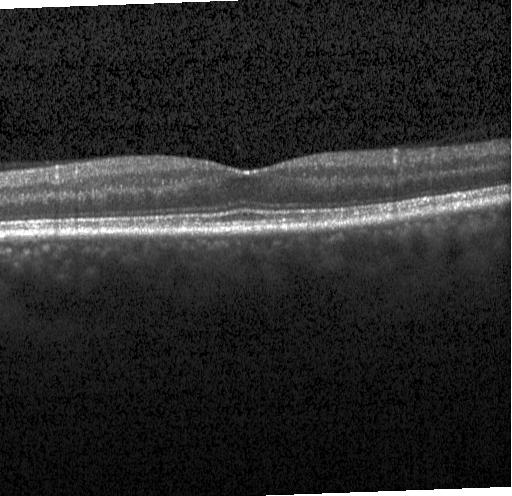

Retinal OCT B-scan · horizontal scan through the fovea · Heidelberg Spectralis OCT system — Dx: neither CNV, DME, nor drusen.